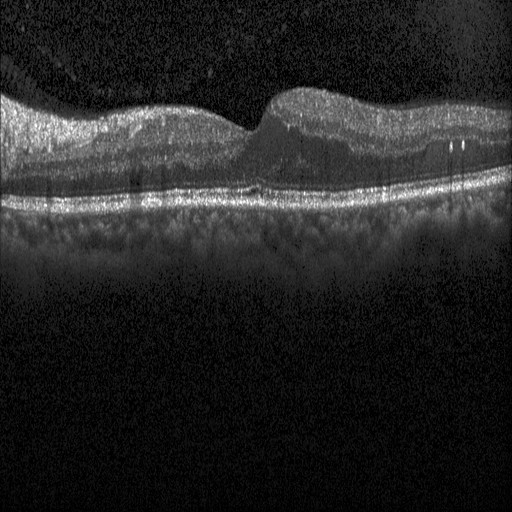

Assessment: diabetic macular edema (DME).